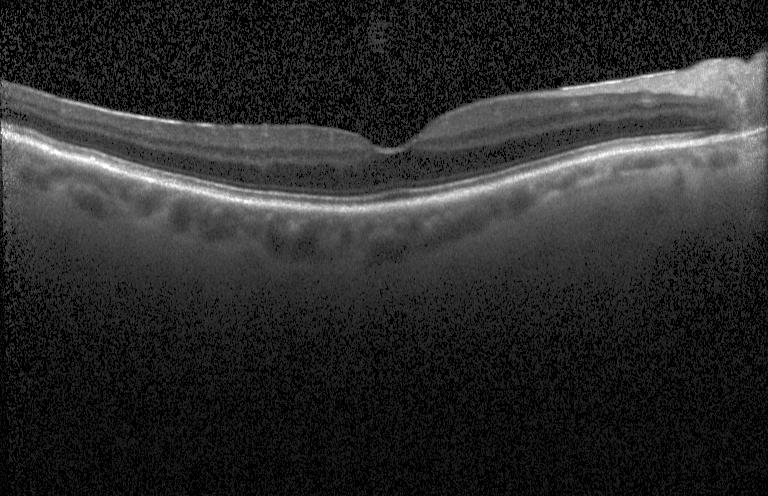

Neither choroidal neovascularization, diabetic macular edema, nor drusen.